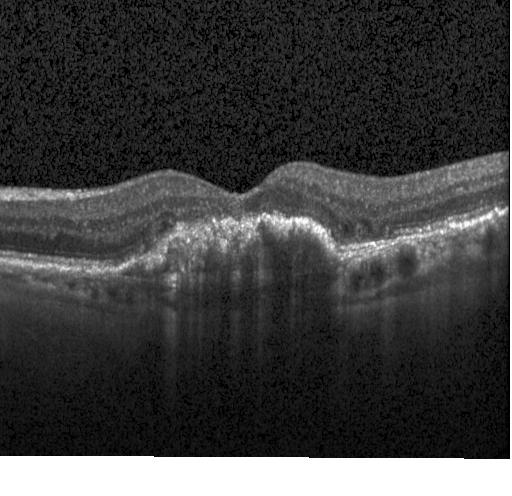 OCT finding: choroidal neovascularization.